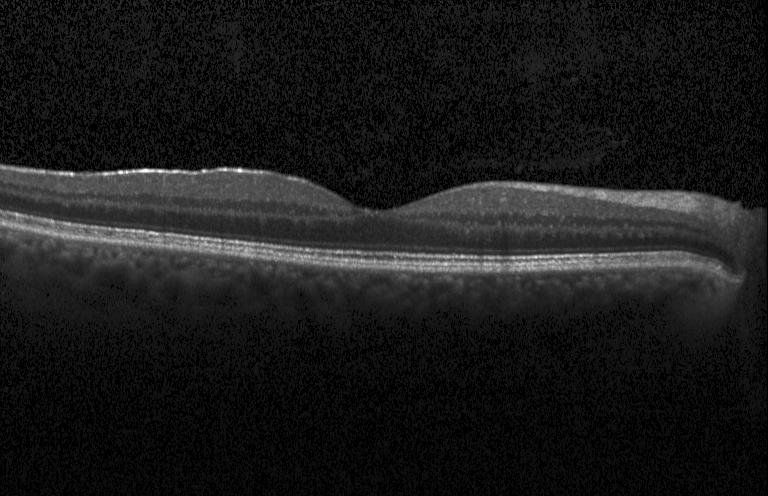

OCT B-scan showing no CNV, DME, or drusen.